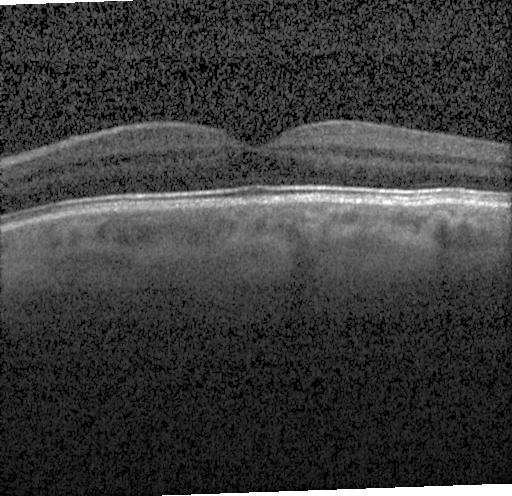
Diagnosis: no choroidal neovascularization, diabetic macular edema, or drusen.